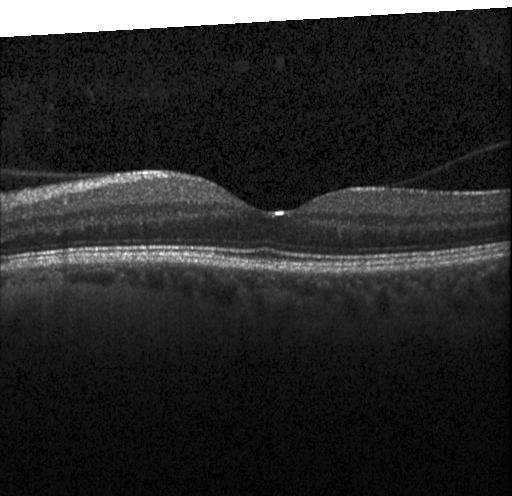 OCT finding: no evidence of CNV, DME, or drusen.